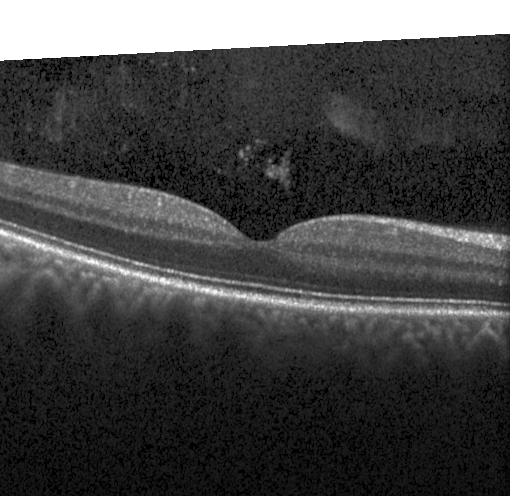 Diagnosis: no choroidal neovascularization, diabetic macular edema, or drusen.